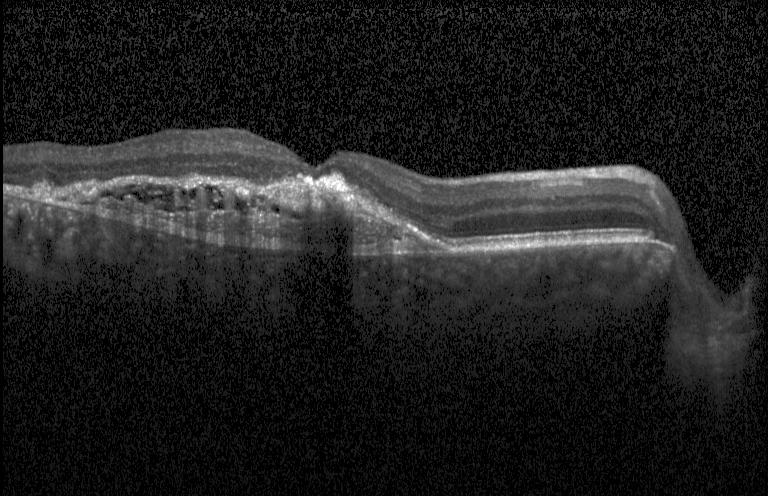 Retinal OCT cross-section. SD-OCT. Horizontal scan through the fovea. Acquired on a Heidelberg Spectralis. Dx: a choroidal neovascular membrane.